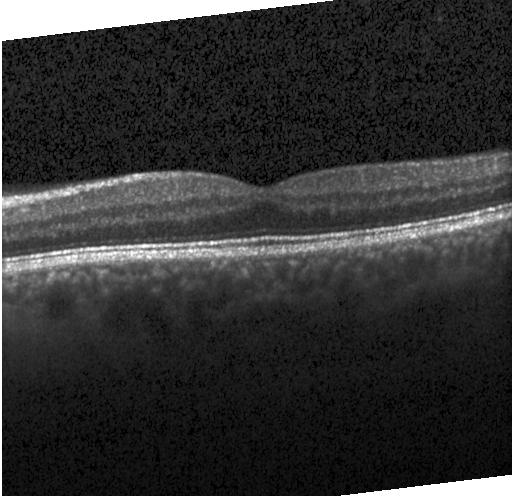 Acquired on a Heidelberg Spectralis. Fovea-centered. Optical coherence tomography scan. SD-OCT
Macular OCT: neither choroidal neovascularization, diabetic macular edema, nor drusen.